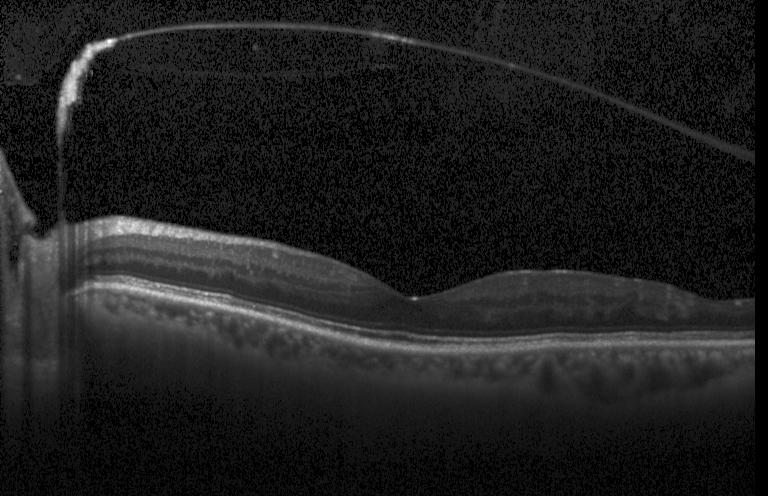
Centered on the fovea, OCT line scan, spectral-domain OCT, Heidelberg Spectralis OCT system. Diagnosis: neither CNV, DME, nor drusen.